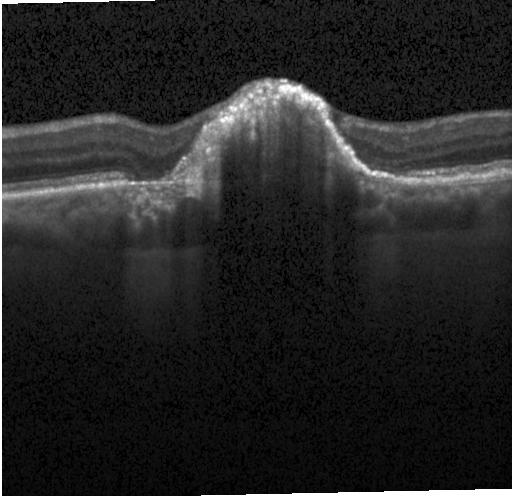

Macular OCT: a choroidal neovascular membrane.